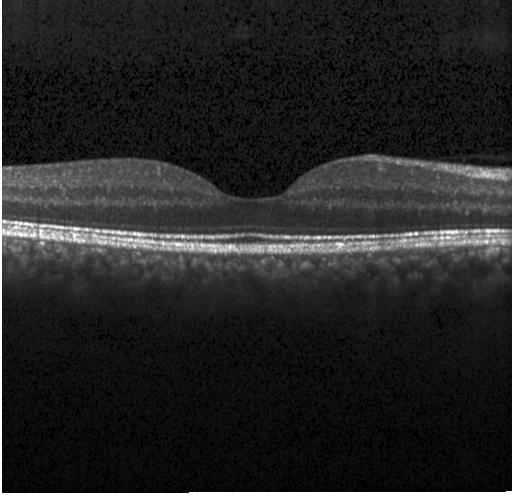

OCT B-scan · instrument: Heidelberg Spectralis · SD-OCT · fovea-centered.
OCT finding: no choroidal neovascularization, no diabetic macular edema, and no drusen.